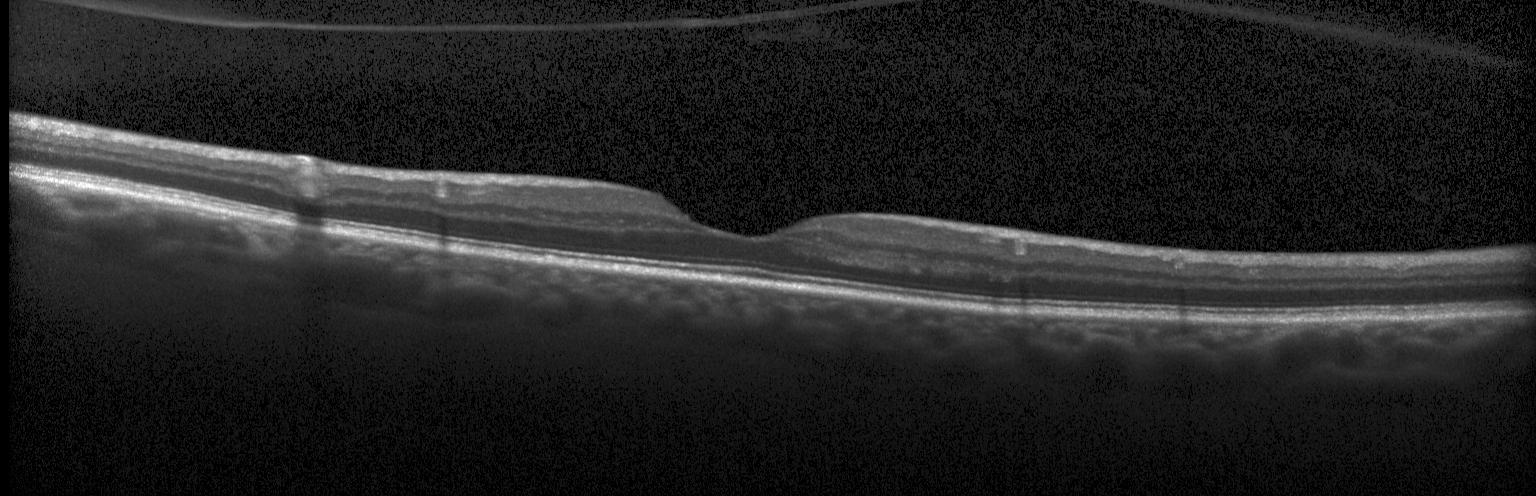
This B-scan demonstrates no choroidal neovascularization, no diabetic macular edema, and no drusen.